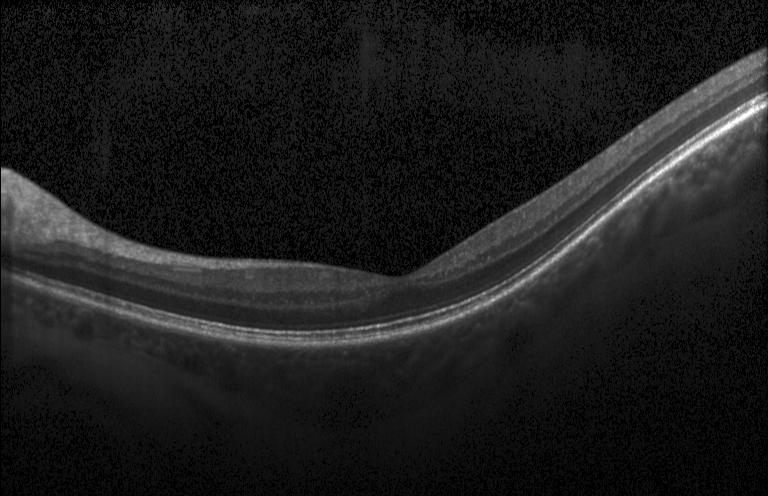 Retinal OCT B-scan; acquired on a Heidelberg Spectralis — Impression: no evidence of choroidal neovascularization, diabetic macular edema, or drusen.